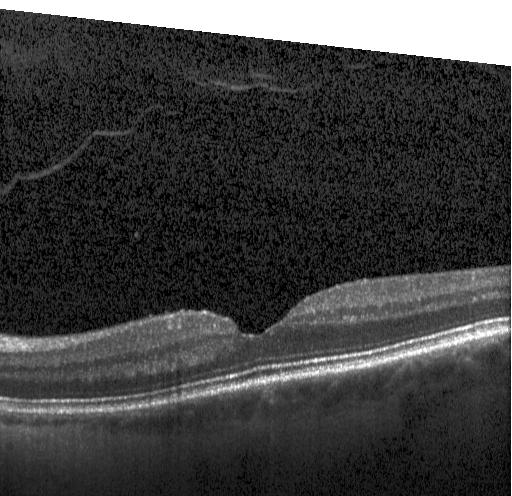

Macular scan. Spectral-domain OCT. Heidelberg Spectralis. Optical coherence tomography B-scan — OCT finding: neither CNV, DME, nor drusen.